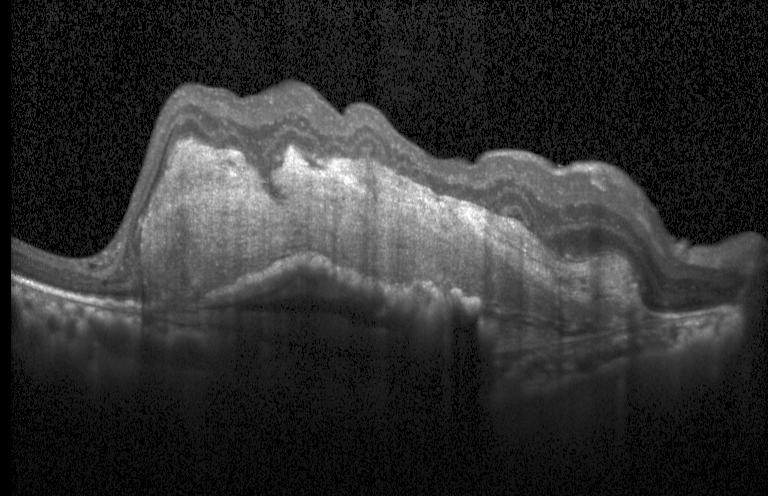 Retinal OCT B-scan. Acquired on a Heidelberg Spectralis. Macular scan — Diagnosis: CNV.